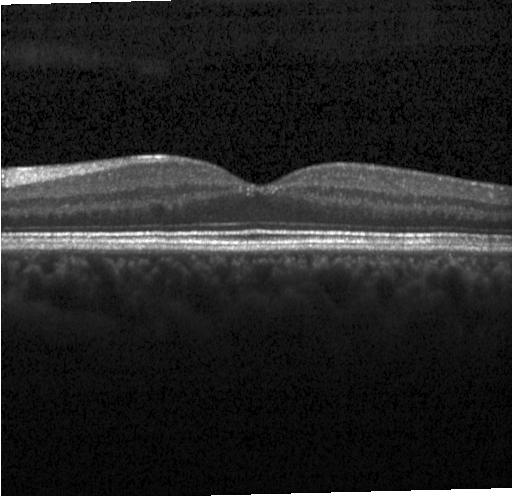 OCT B-scan
The scan shows no evidence of CNV, DME, or drusen.